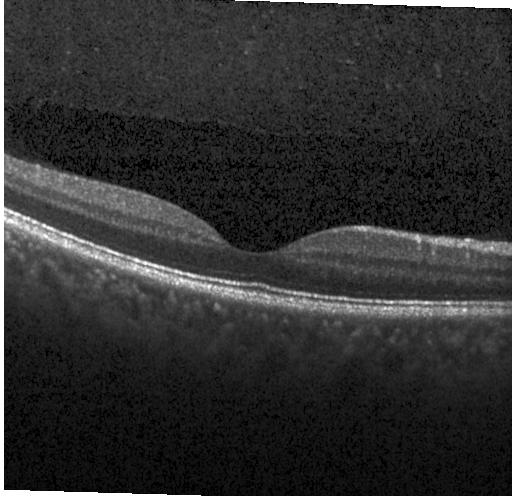
Acquired on a Heidelberg Spectralis · retinal OCT cross-section · fovea-centered · SD-OCT — Dx: no choroidal neovascularization, diabetic macular edema, or drusen.